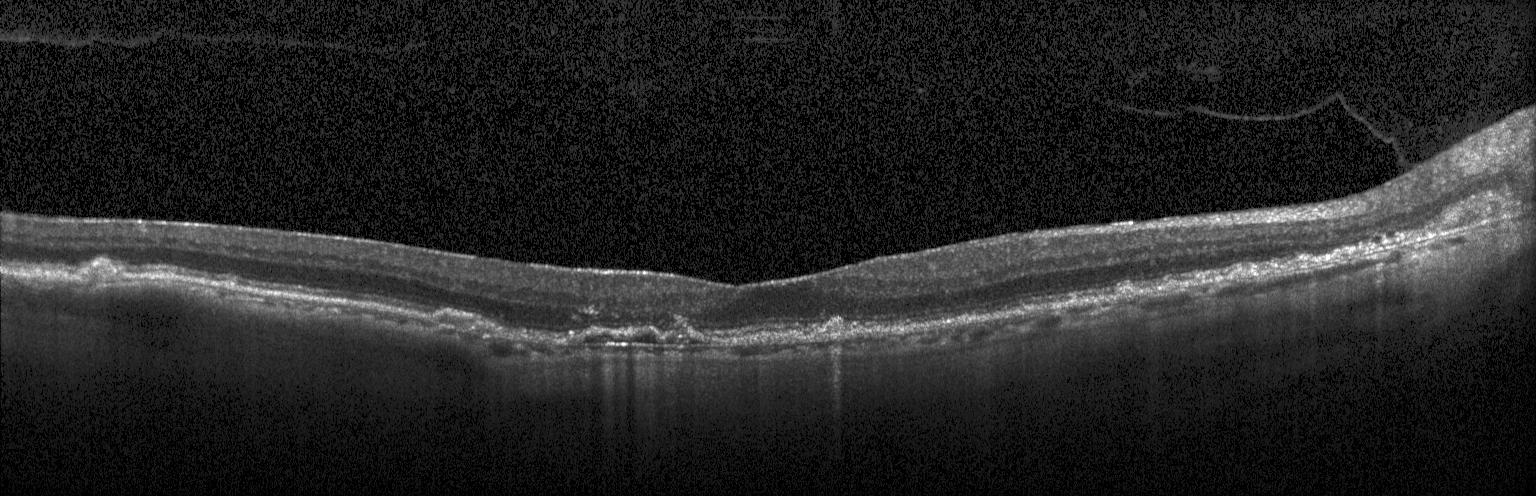
Optical coherence tomography scan. Macular scan. Acquired on a Heidelberg Spectralis. SD-OCT. Dx: a choroidal neovascular membrane.